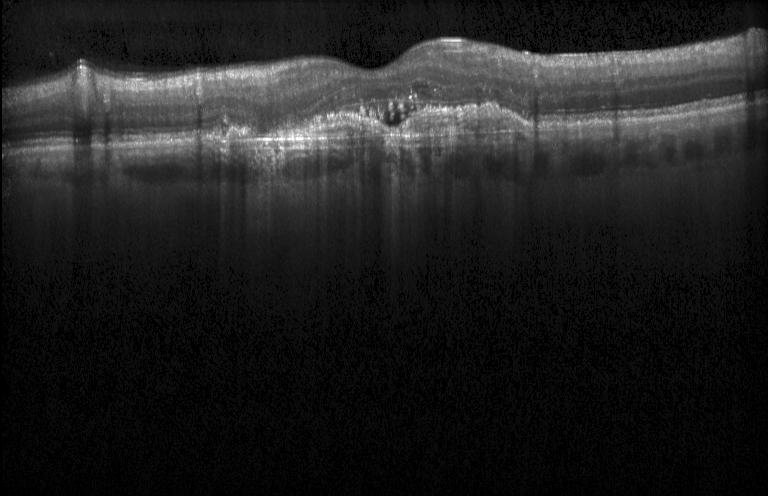
Heidelberg Spectralis OCT system · through the macula · OCT line scan. This B-scan demonstrates CNV.